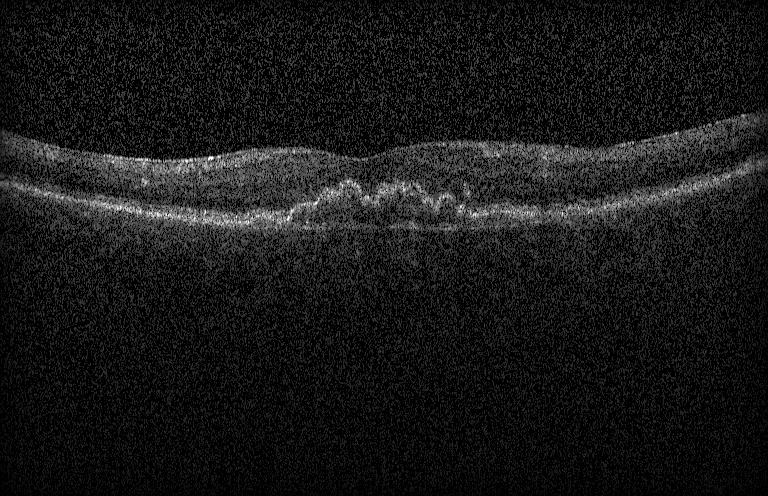
Macular OCT: a choroidal neovascular membrane.